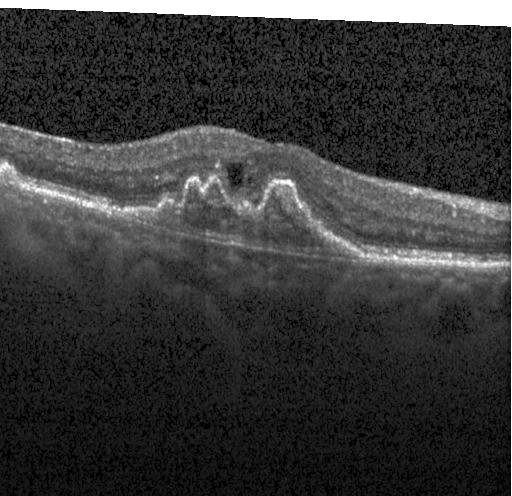

Heidelberg Spectralis OCT system. Retinal OCT cross-section — This B-scan demonstrates a choroidal neovascular membrane.